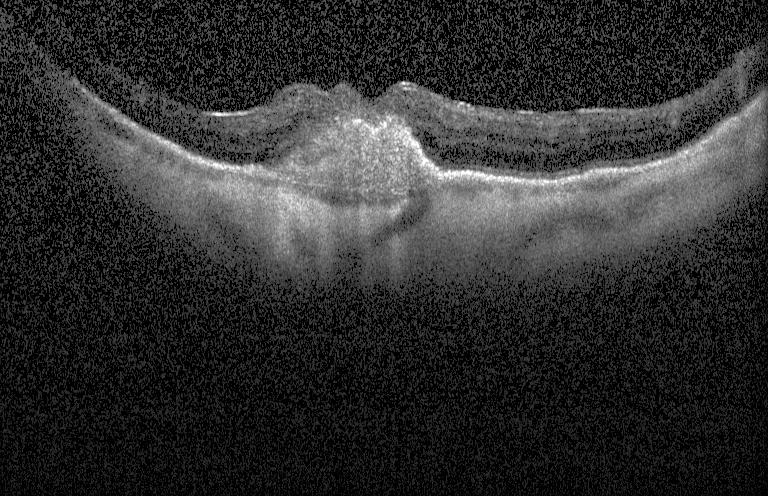

Macular OCT: a choroidal neovascular membrane.